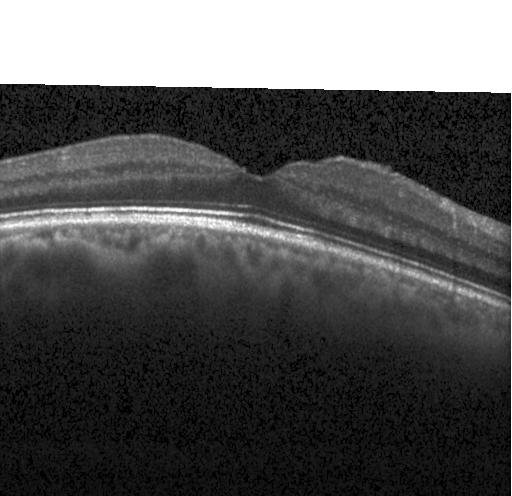

Centered on the fovea. Spectral-domain OCT. OCT line scan. Heidelberg Spectralis.
OCT finding: neither choroidal neovascularization, diabetic macular edema, nor drusen.